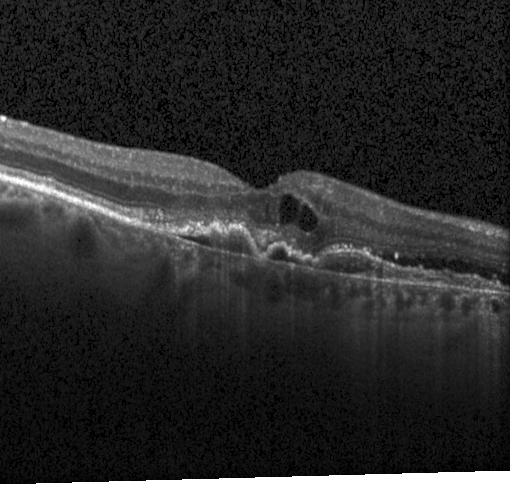

Diagnosis: choroidal neovascularization (CNV).